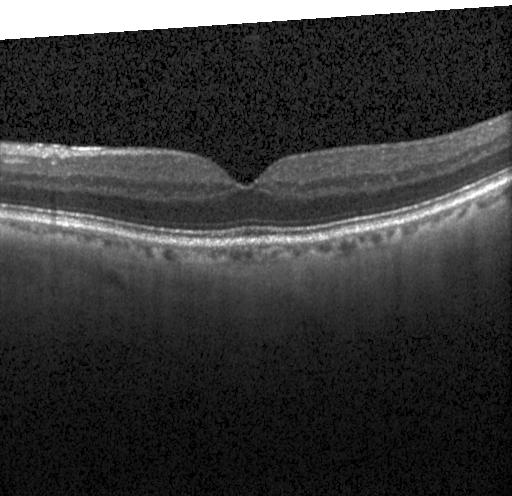

Heidelberg Spectralis OCT system. OCT line scan. Horizontal scan through the fovea. SD-OCT. Dx: no choroidal neovascularization, no diabetic macular edema, and no drusen.